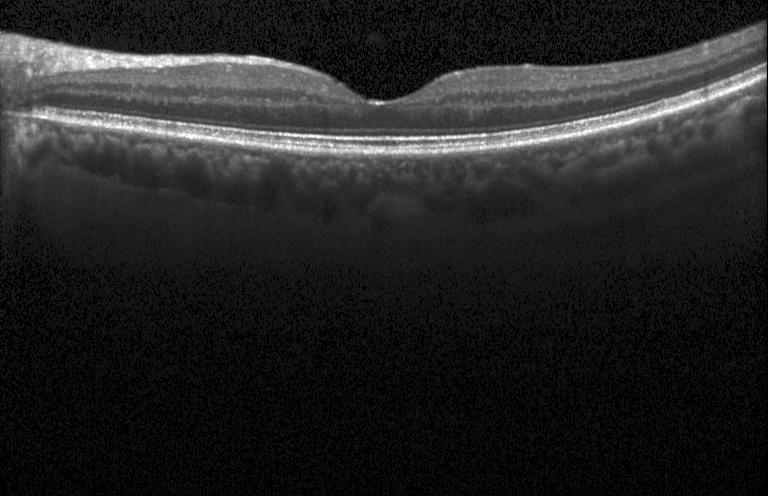
OCT finding: neither CNV, DME, nor drusen.